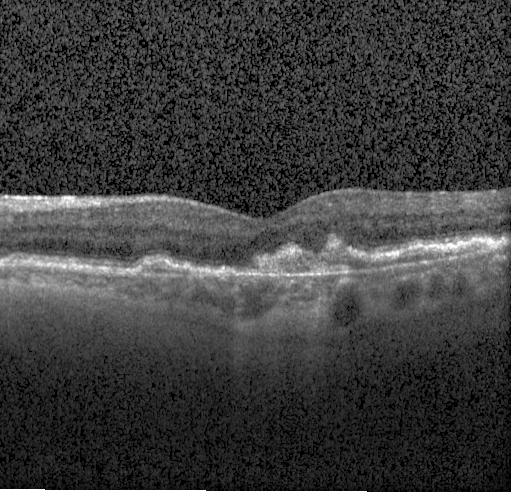
Optical coherence tomography scan. Spectral-domain optical coherence tomography. Heidelberg Spectralis OCT system.
Choroidal neovascularization (CNV).